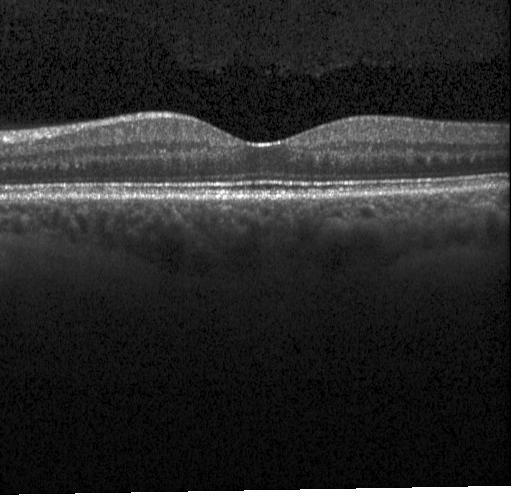

OCT finding: neither choroidal neovascularization, diabetic macular edema, nor drusen.